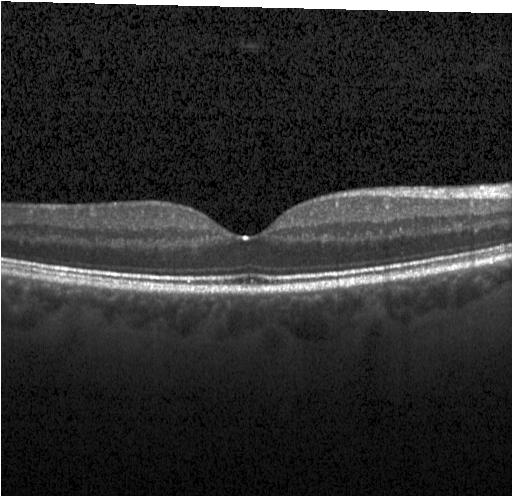 Optical coherence tomography B-scan.
Impression: no evidence of choroidal neovascularization, diabetic macular edema, or drusen.